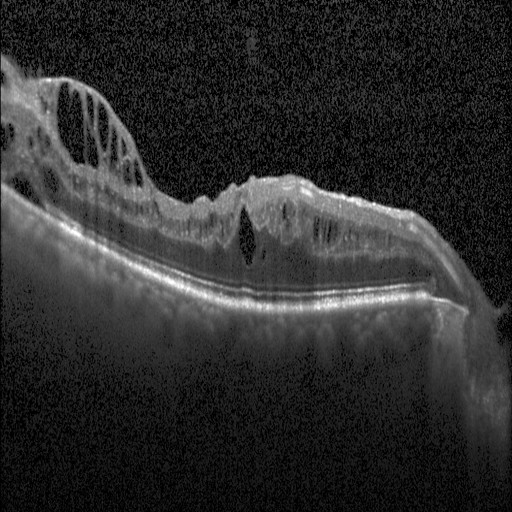 OCT line scan · spectral-domain OCT — Diagnosis: diabetic macular edema.